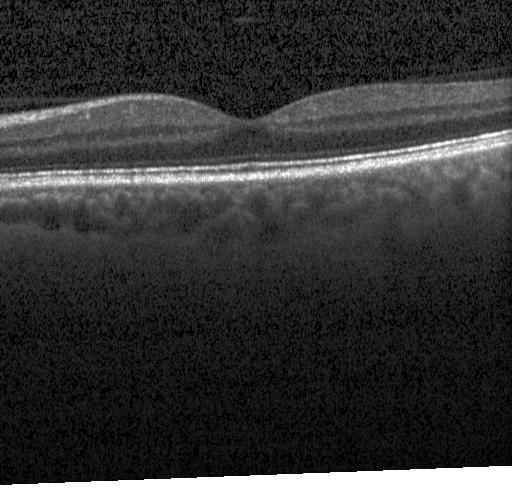
Macular OCT: no choroidal neovascularization, diabetic macular edema, or drusen.